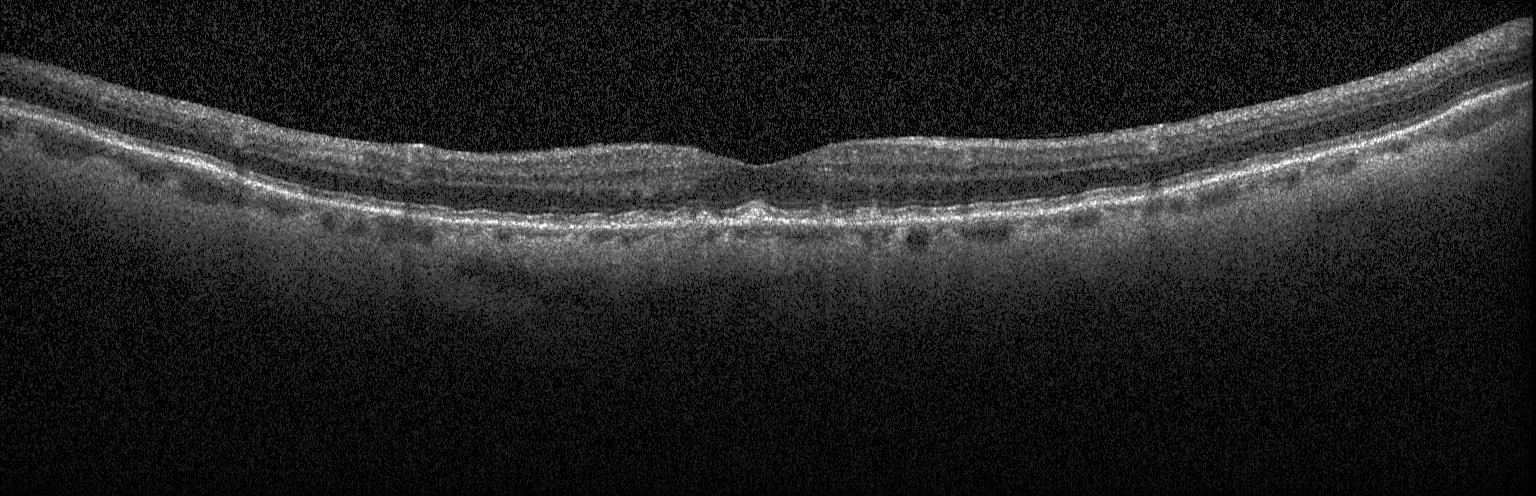

OCT B-scan showing drusen.